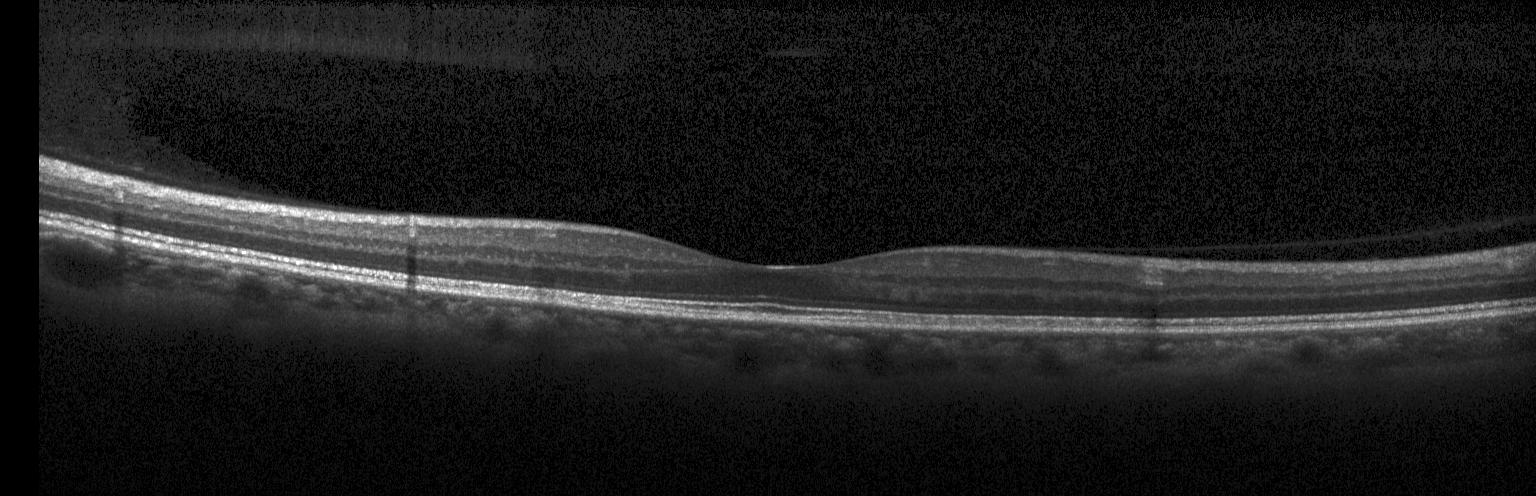 Spectral-domain OCT B-scan: neither choroidal neovascularization, diabetic macular edema, nor drusen.